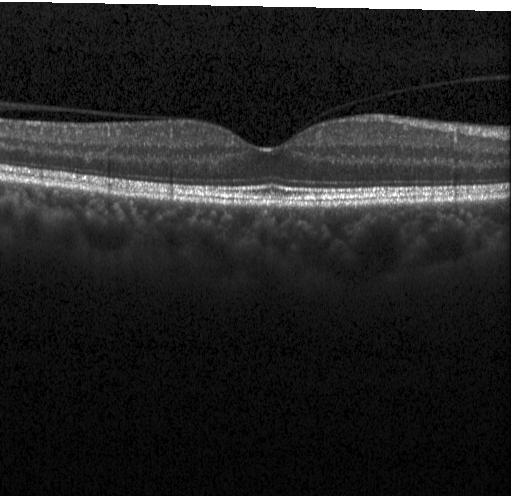

Retinal OCT cross-section
Impression: neither choroidal neovascularization, diabetic macular edema, nor drusen.